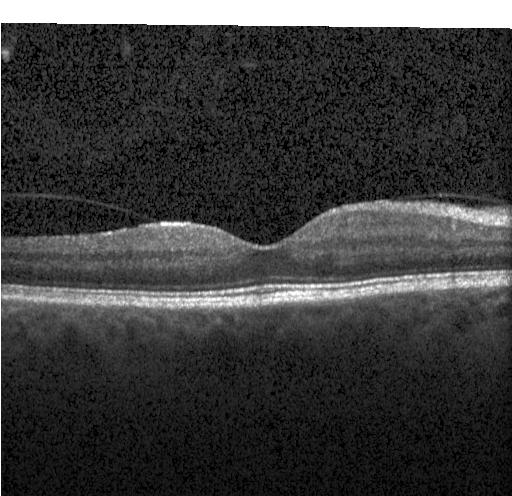 OCT B-scan — Diagnosis: neither choroidal neovascularization, diabetic macular edema, nor drusen.